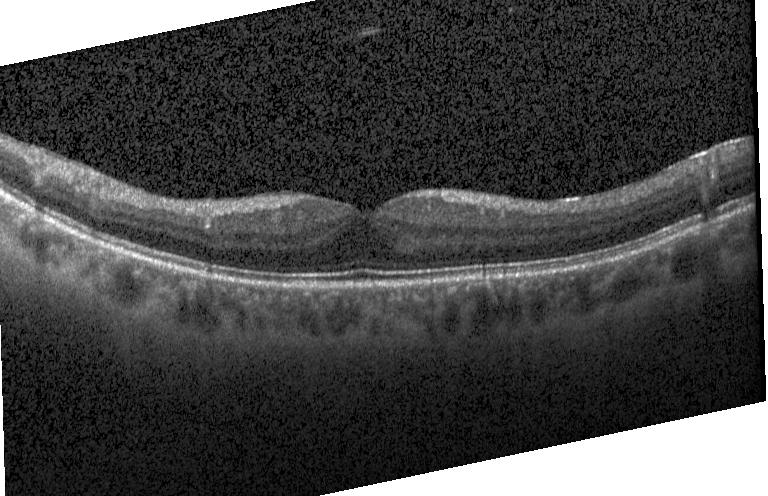

Spectral-domain OCT; instrument: Heidelberg Spectralis; retinal OCT B-scan. This B-scan demonstrates no choroidal neovascularization, diabetic macular edema, or drusen.